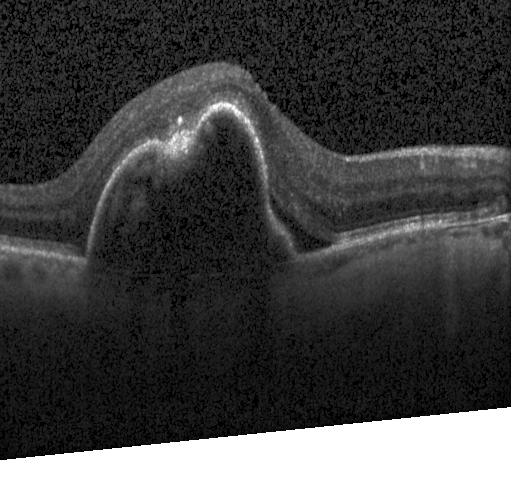

Assessment: choroidal neovascularization.